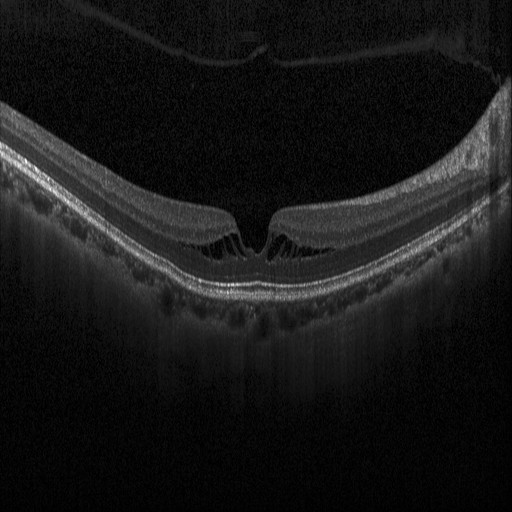 Centered on the fovea · Heidelberg Spectralis OCT system · SD-OCT · retinal OCT cross-section. Finding: diabetic macular edema (DME).